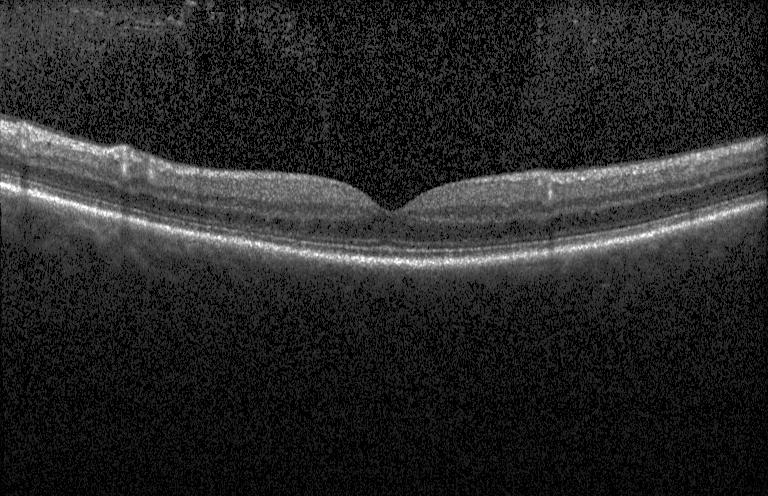

OCT finding: neither choroidal neovascularization, diabetic macular edema, nor drusen.